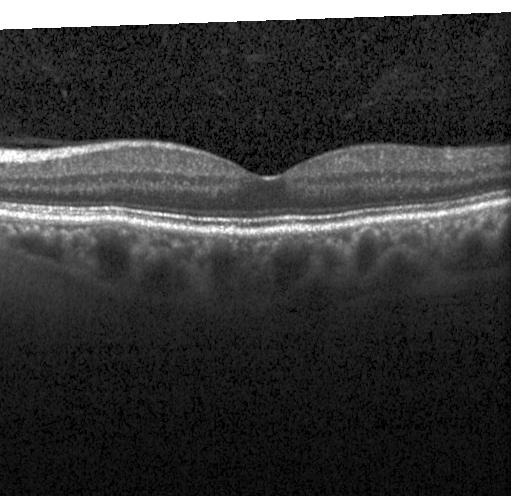

The scan shows neither choroidal neovascularization, diabetic macular edema, nor drusen.